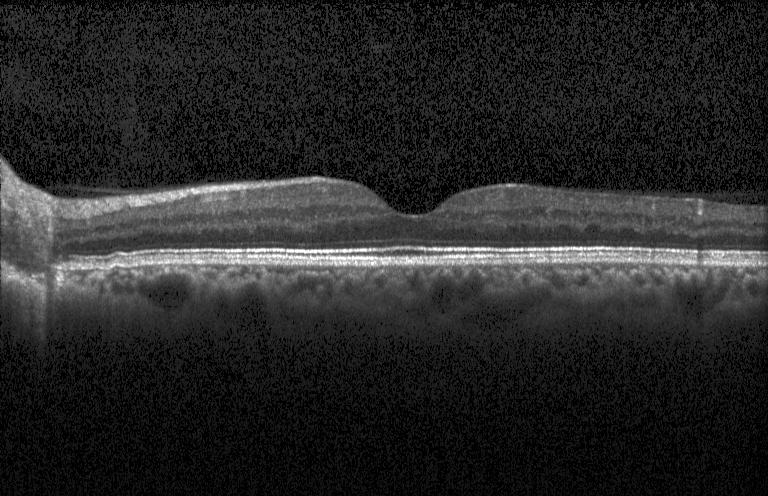

Retinal OCT cross-section. Assessment: no evidence of CNV, DME, or drusen.